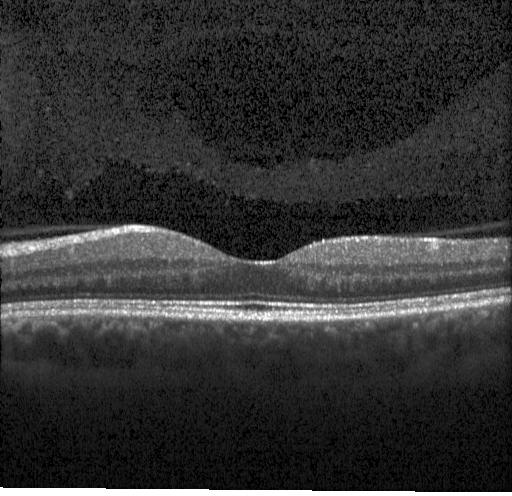

Optical coherence tomography scan. Horizontal scan through the fovea. Acquired on a Heidelberg Spectralis — Finding: no evidence of choroidal neovascularization, diabetic macular edema, or drusen.